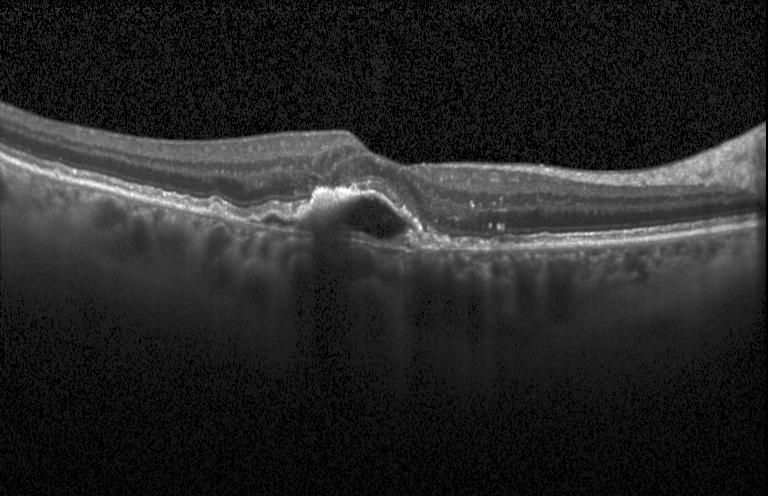 OCT B-scan showing choroidal neovascularization.